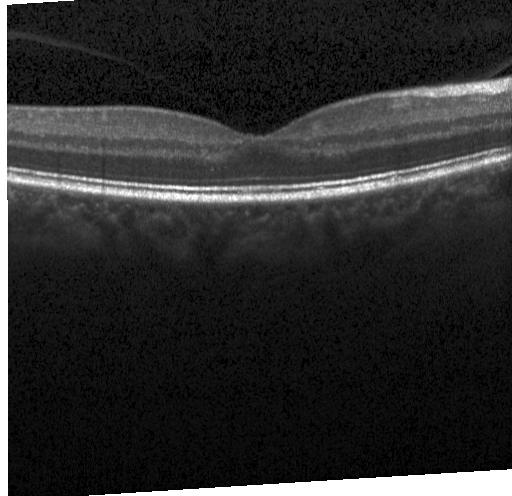 Retinal OCT cross-section · horizontal scan through the fovea · Heidelberg Spectralis OCT system · spectral-domain OCT — Assessment: no evidence of choroidal neovascularization, diabetic macular edema, or drusen.